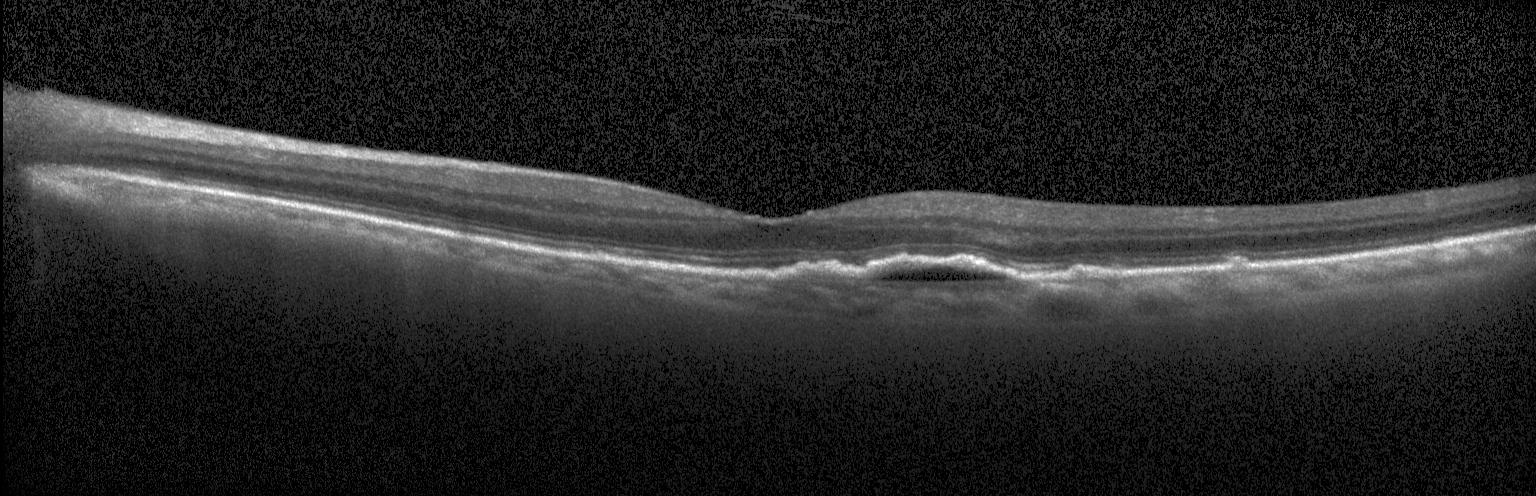

OCT finding: choroidal neovascularization.